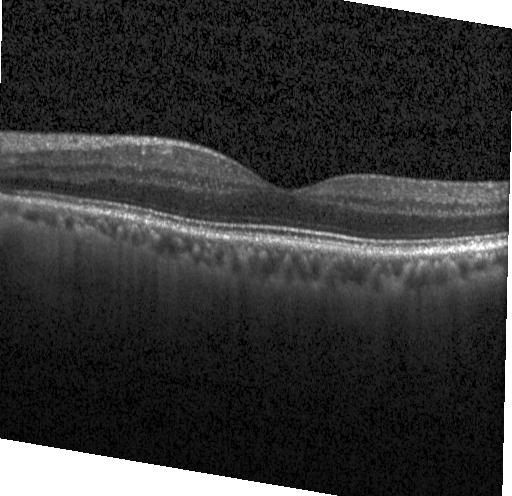

Finding: no evidence of choroidal neovascularization, diabetic macular edema, or drusen.